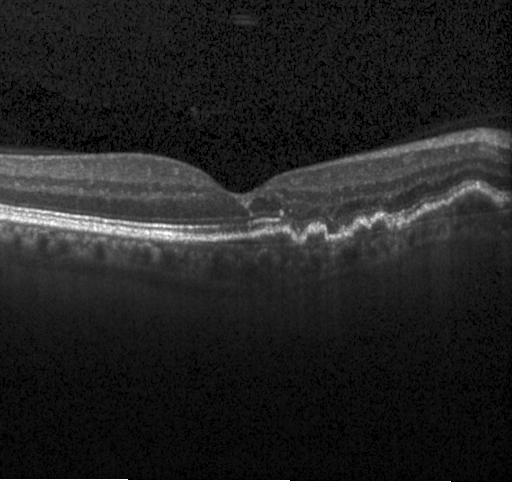 Optical coherence tomography scan — This B-scan demonstrates CNV.